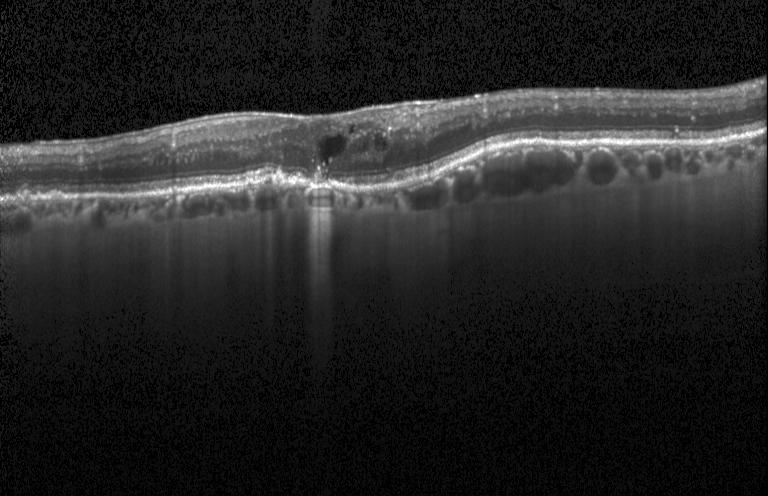 Optical coherence tomography B-scan
Choroidal neovascularization.